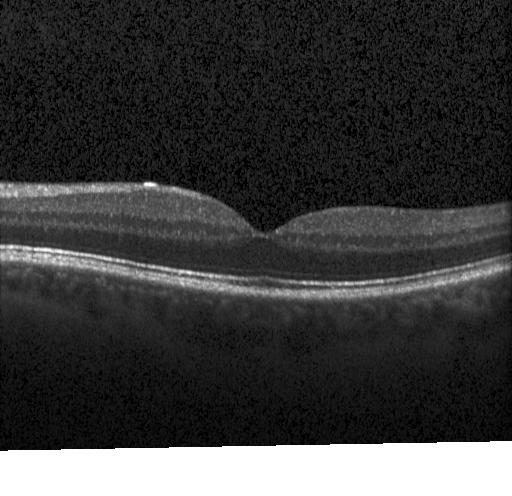 OCT scan showing no choroidal neovascularization, no diabetic macular edema, and no drusen.